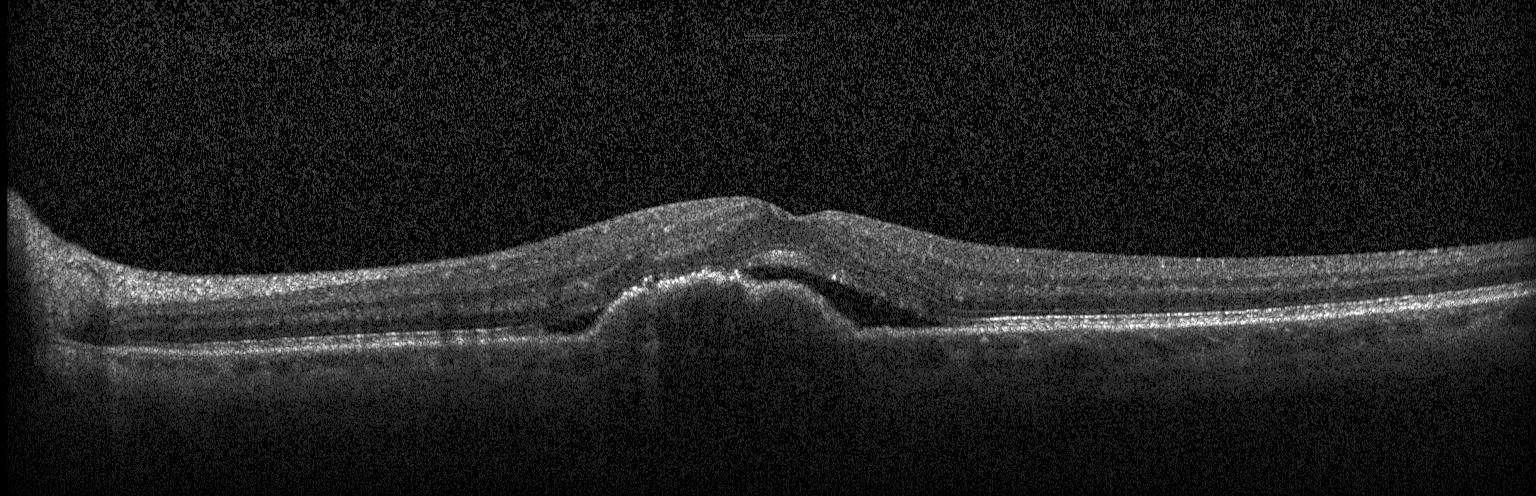 Spectral-domain optical coherence tomography. Optical coherence tomography B-scan. Instrument: Heidelberg Spectralis.
Impression: choroidal neovascularization.